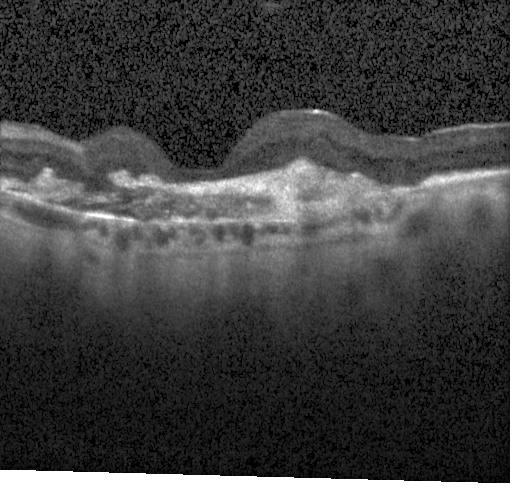 Finding: a choroidal neovascular membrane.